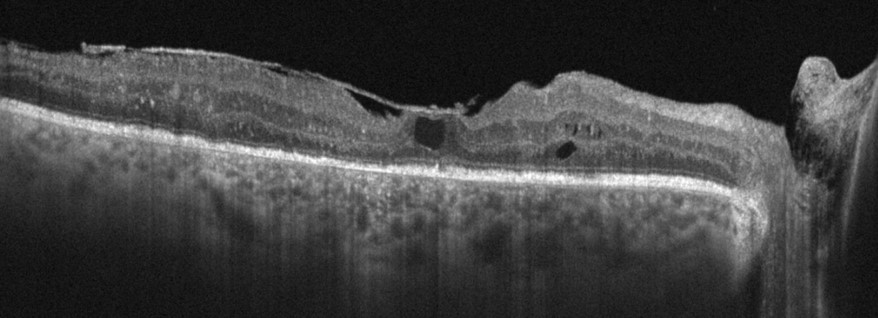

Retinal OCT cross-section
The scan shows DME.